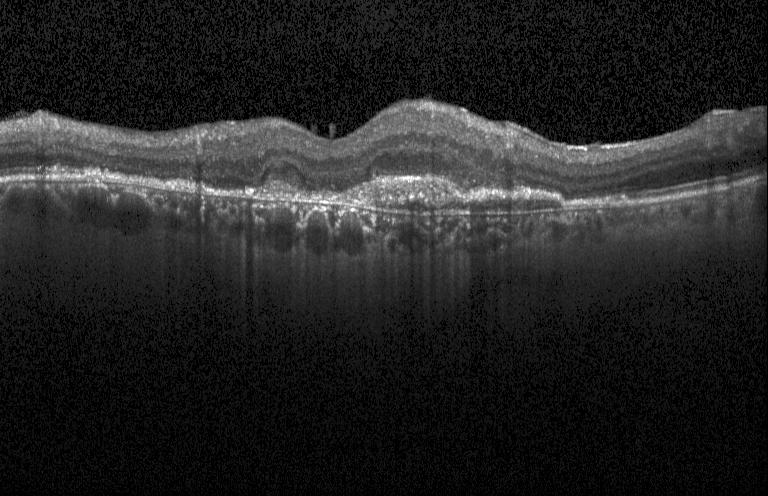

OCT B-scan. The scan shows a choroidal neovascular membrane.